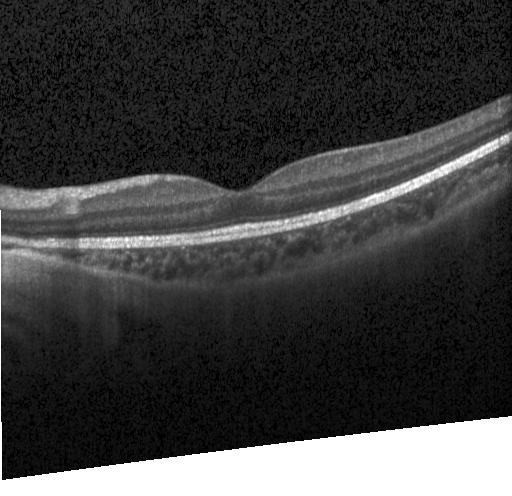

OCT B-scan showing no CNV, no DME, and no drusen.